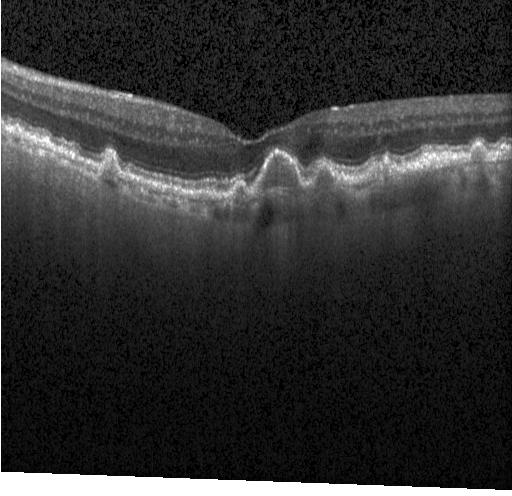 Centered on the fovea. Acquired on a Heidelberg Spectralis. Optical coherence tomography B-scan. SD-OCT
Impression: drusen.